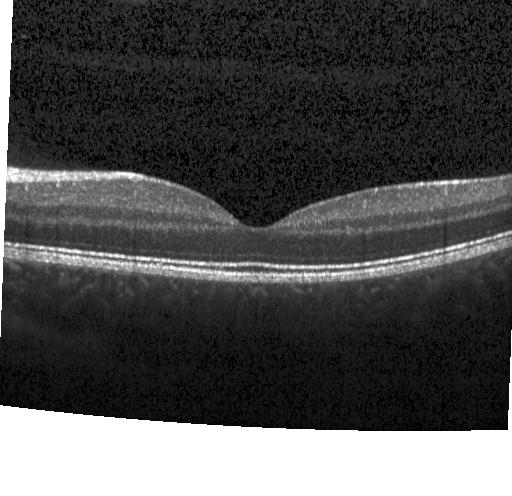 OCT finding: no choroidal neovascularization, diabetic macular edema, or drusen.